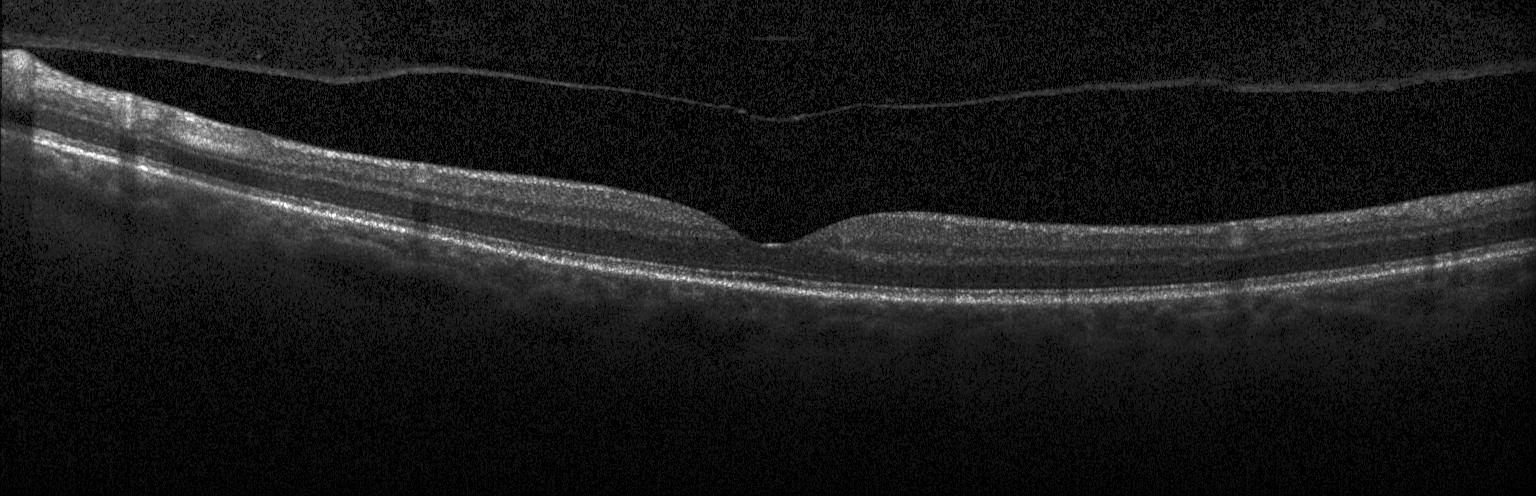

The scan shows neither CNV, DME, nor drusen.